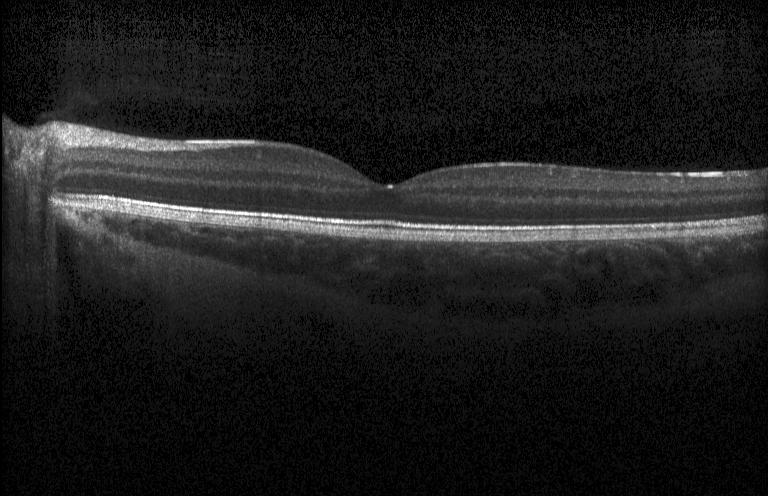

Optical coherence tomography scan; Heidelberg Spectralis; SD-OCT. Impression: no CNV, DME, or drusen.